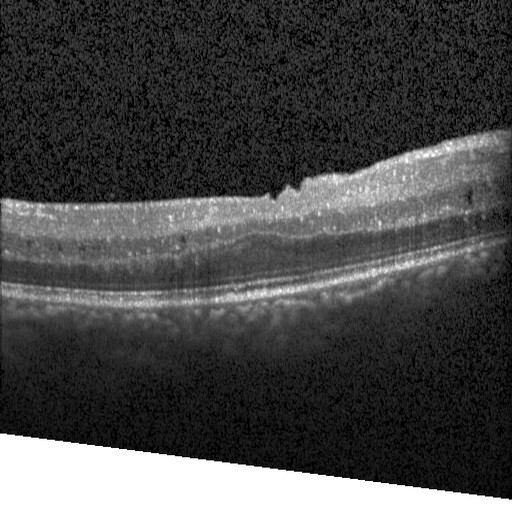

Macular OCT: diabetic macular edema.